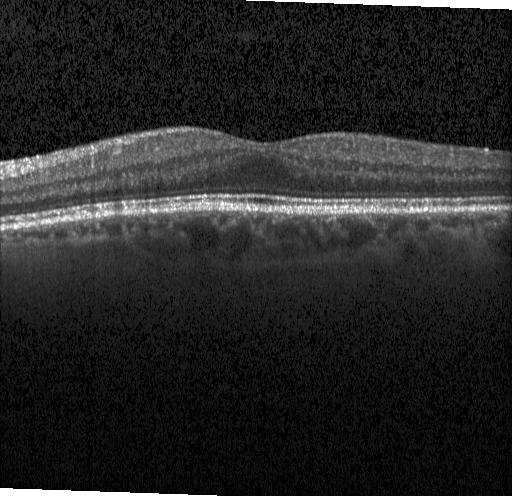
OCT line scan, horizontal scan through the fovea, SD-OCT, Heidelberg Spectralis.
Macular OCT: no evidence of choroidal neovascularization, diabetic macular edema, or drusen.